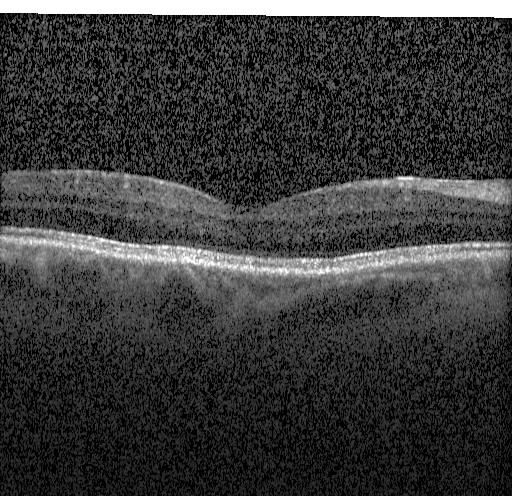
Heidelberg Spectralis; fovea-centered; spectral-domain optical coherence tomography; optical coherence tomography scan. Diagnosis: neither CNV, DME, nor drusen.